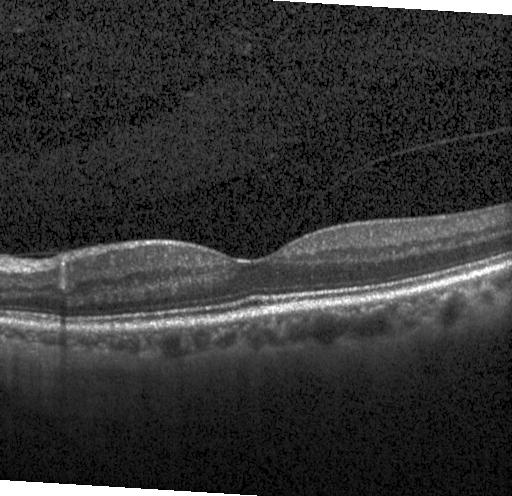
Heidelberg Spectralis OCT system, retinal OCT cross-section, spectral-domain optical coherence tomography, horizontal scan through the fovea — No choroidal neovascularization, diabetic macular edema, or drusen.